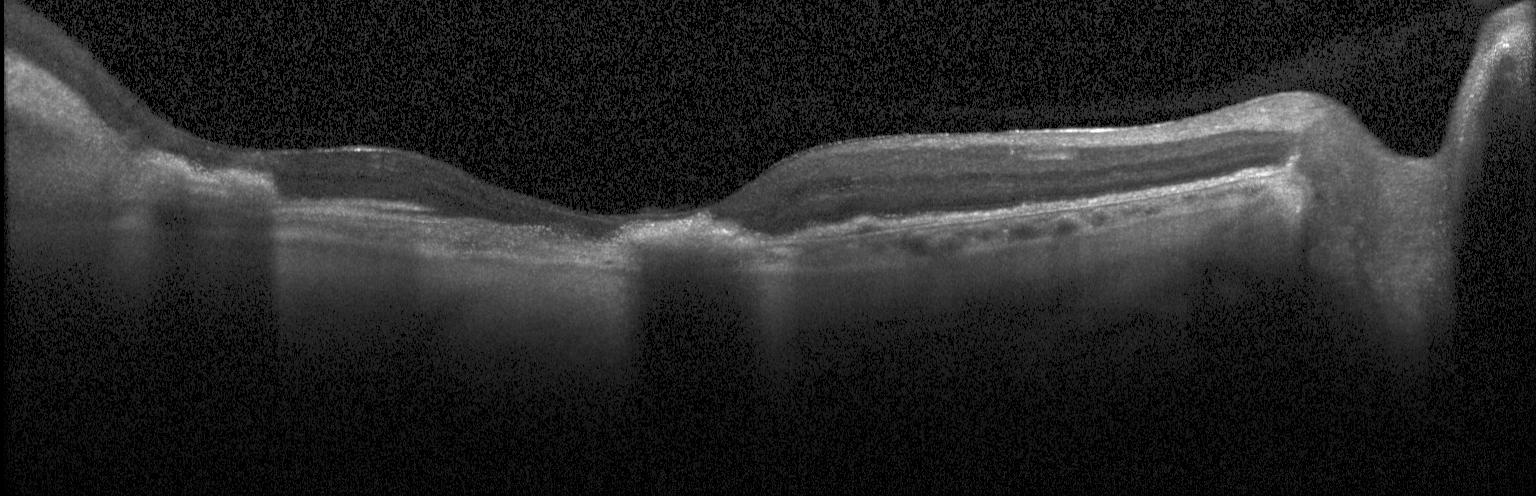

OCT B-scan showing choroidal neovascularization (CNV).